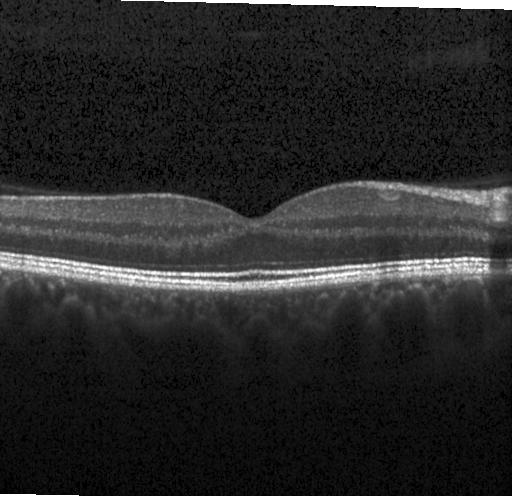
OCT line scan; spectral-domain OCT; fovea-centered; Heidelberg Spectralis.
OCT finding: no choroidal neovascularization, no diabetic macular edema, and no drusen.